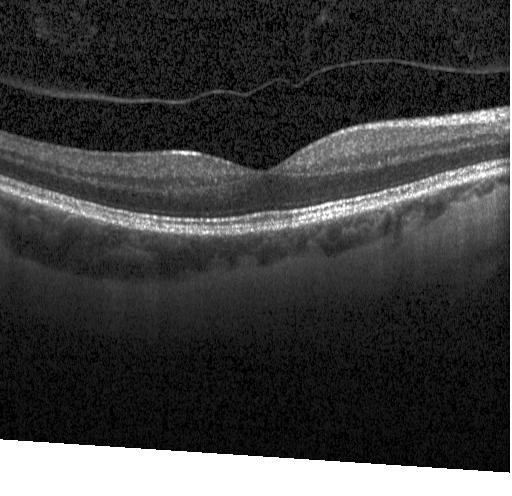 Finding: neither CNV, DME, nor drusen.